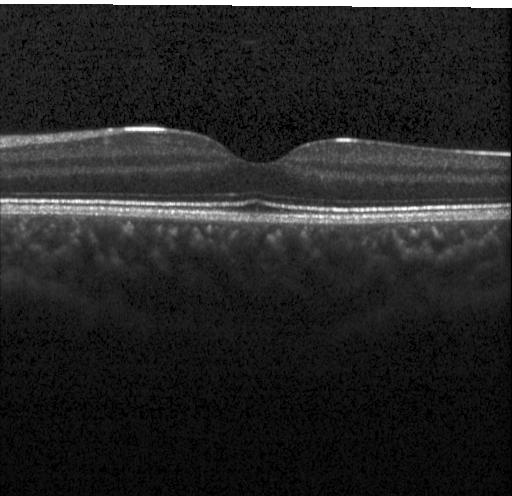 Optical coherence tomography scan. OCT finding: neither choroidal neovascularization, diabetic macular edema, nor drusen.